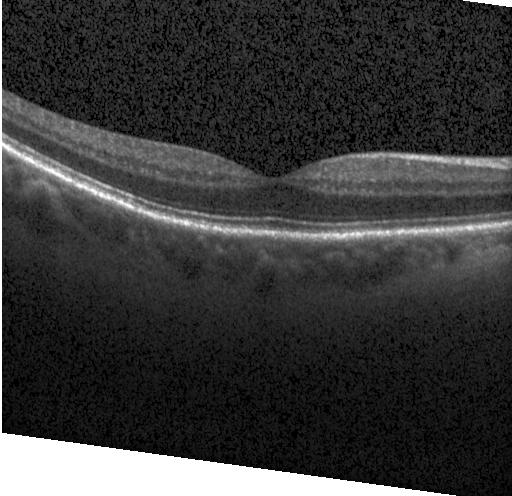
OCT line scan · horizontal scan through the fovea · spectral-domain OCT · acquired on a Heidelberg Spectralis. Impression: no choroidal neovascularization, diabetic macular edema, or drusen.